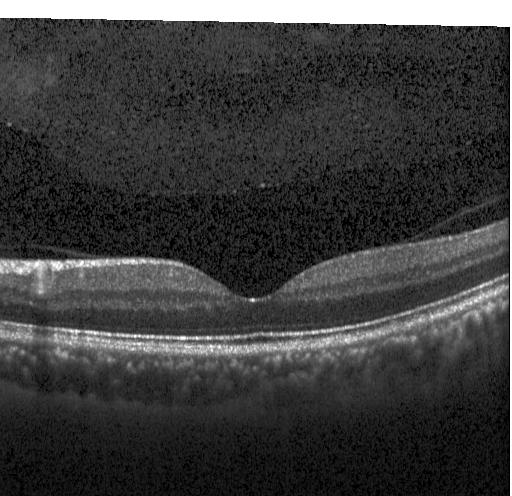

OCT finding: no evidence of choroidal neovascularization, diabetic macular edema, or drusen.